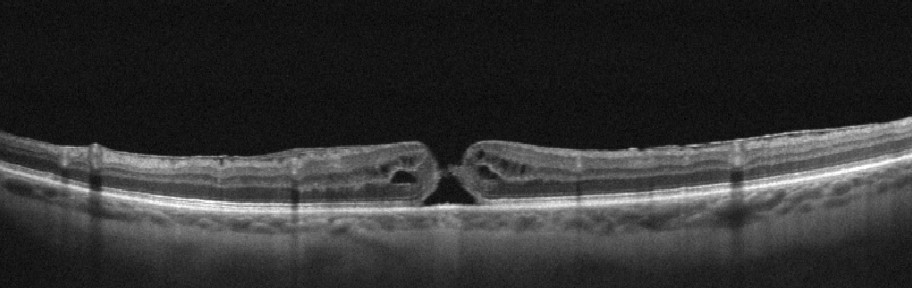 Retinal OCT cross-section showing vitreomacular interface disease (VID).